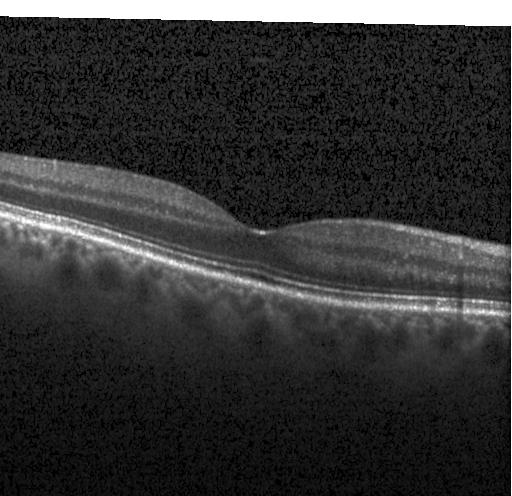 Retinal OCT cross-section · fovea-centered — Finding: no evidence of choroidal neovascularization, diabetic macular edema, or drusen.